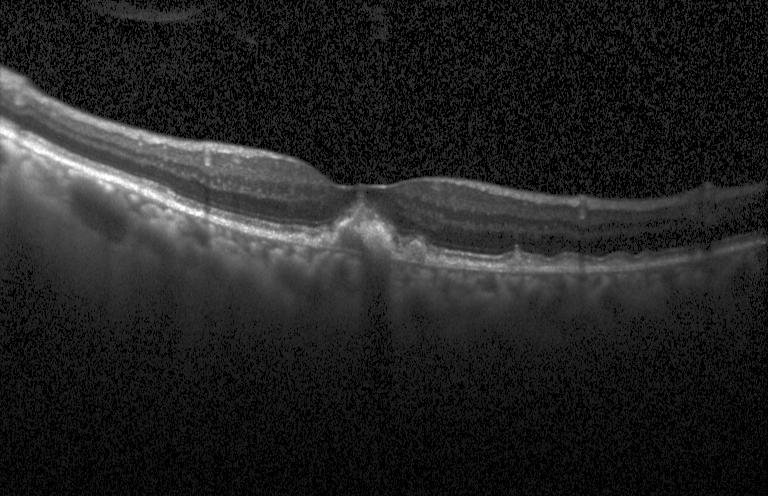

This B-scan demonstrates a choroidal neovascular membrane.